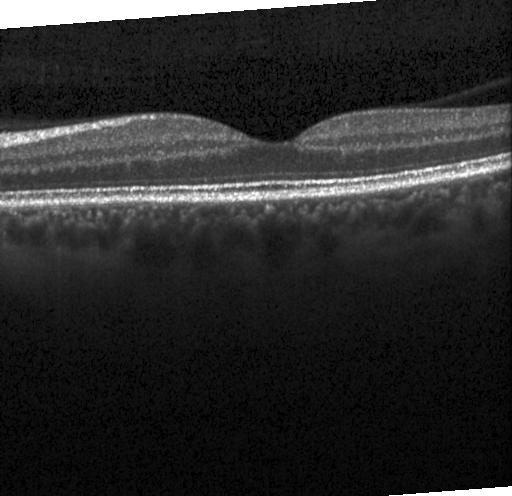 Optical coherence tomography B-scan.
Assessment: no evidence of choroidal neovascularization, diabetic macular edema, or drusen.